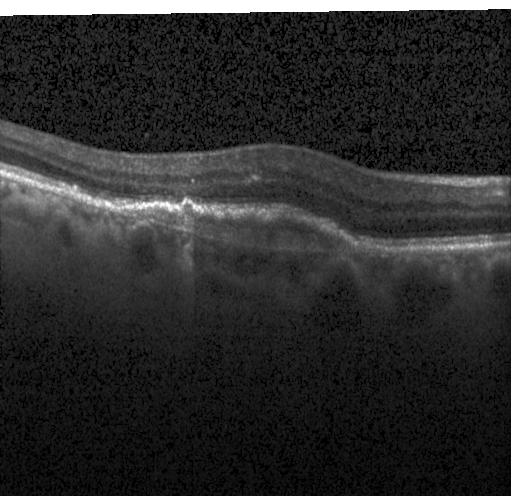

This B-scan demonstrates a choroidal neovascular membrane.